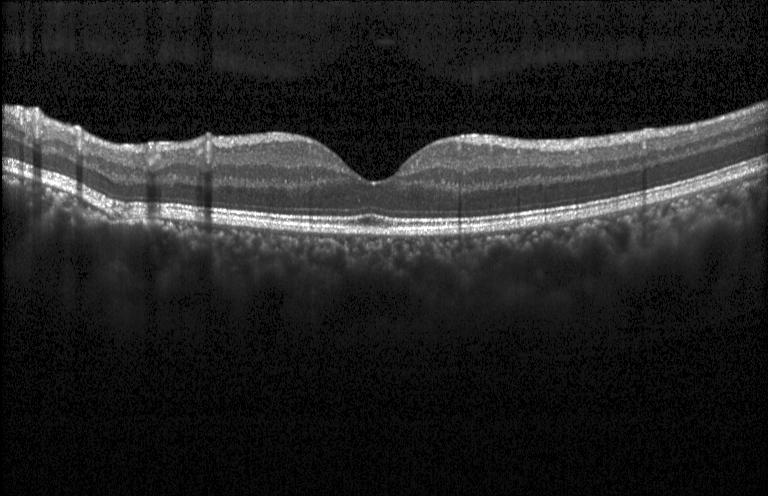
Heidelberg Spectralis OCT system; retinal OCT B-scan. Dx: no CNV, no DME, and no drusen.